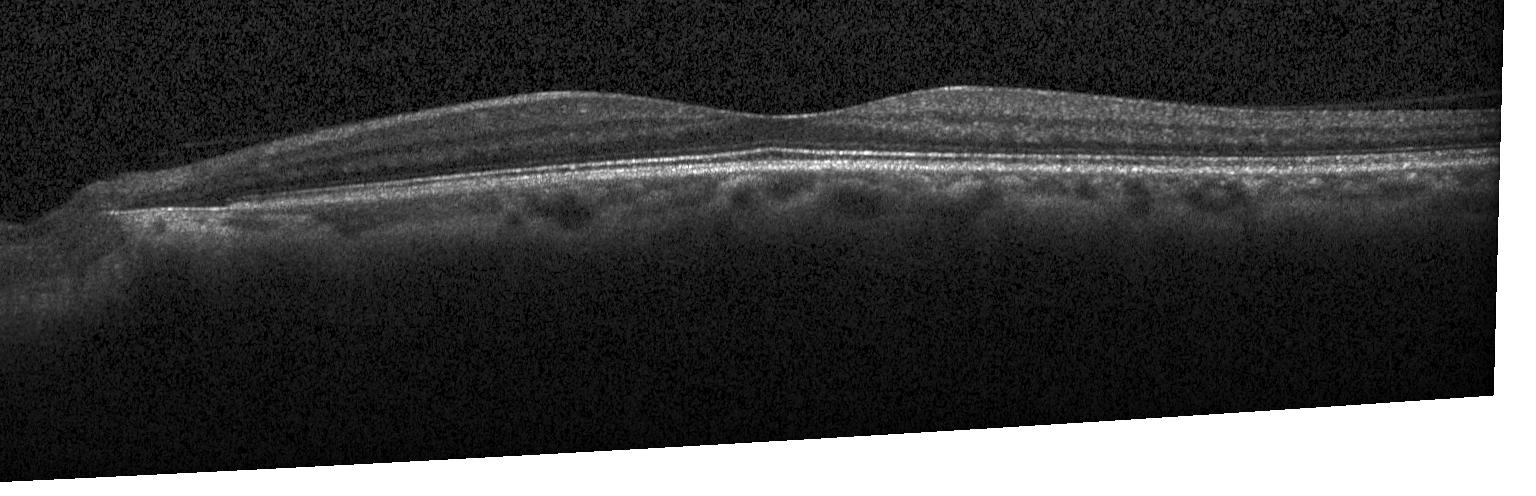 Spectral-domain optical coherence tomography; optical coherence tomography B-scan; centered on the fovea. Impression: no CNV, DME, or drusen.